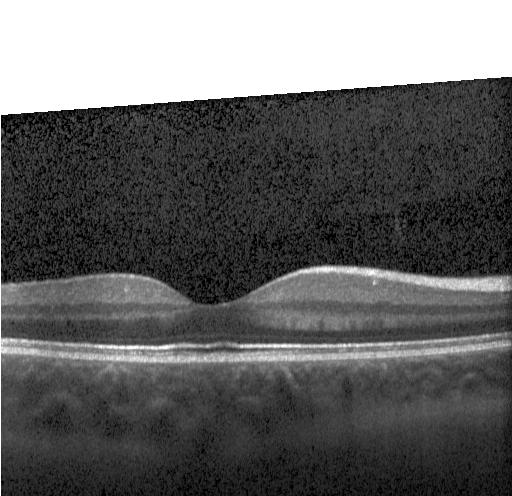
Retinal OCT cross-section showing no choroidal neovascularization, no diabetic macular edema, and no drusen.